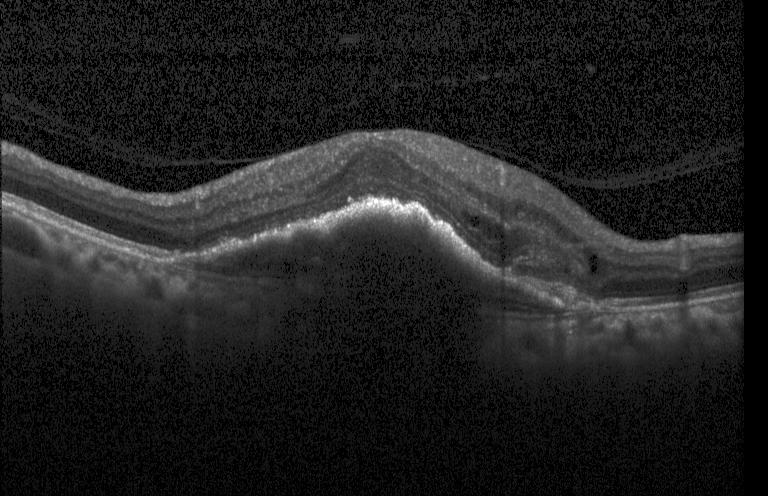

Retinal OCT B-scan — Impression: a choroidal neovascular membrane.